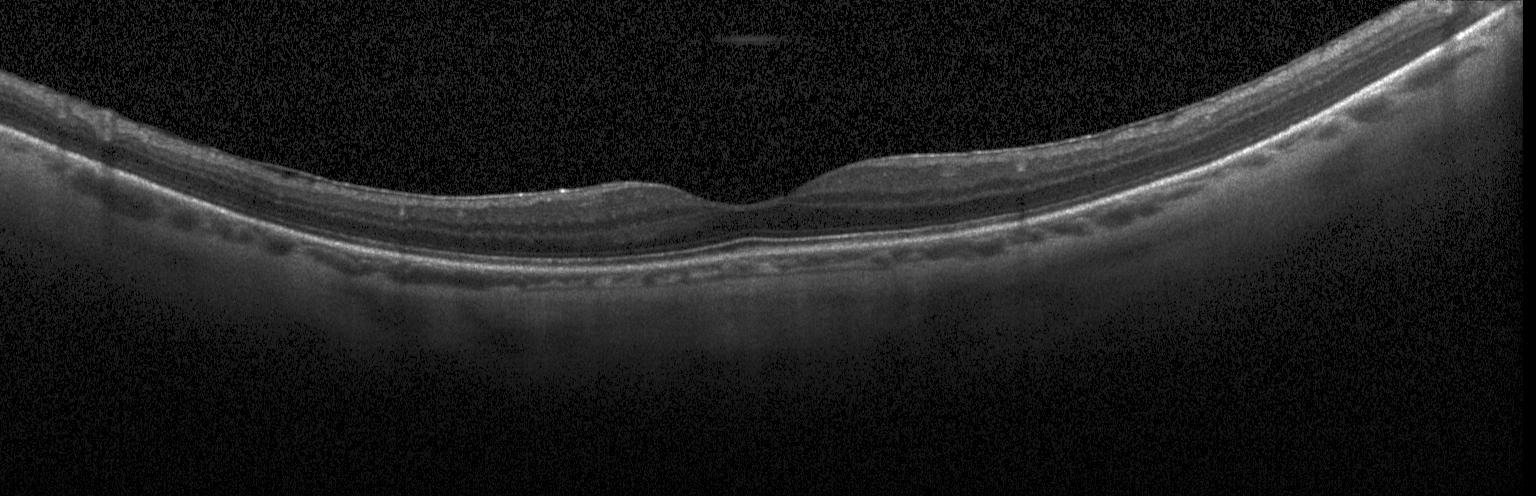

Heidelberg Spectralis, optical coherence tomography B-scan.
Diagnosis: no choroidal neovascularization, no diabetic macular edema, and no drusen.